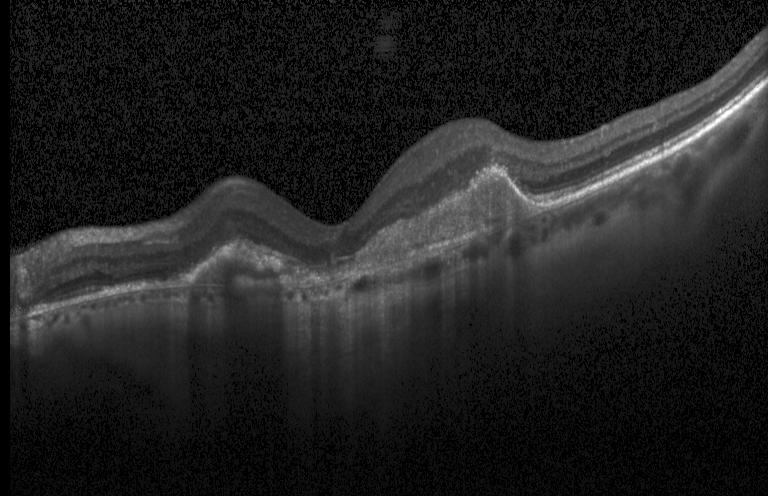

Heidelberg Spectralis · spectral-domain OCT · OCT B-scan · fovea-centered
Impression: a choroidal neovascular membrane.